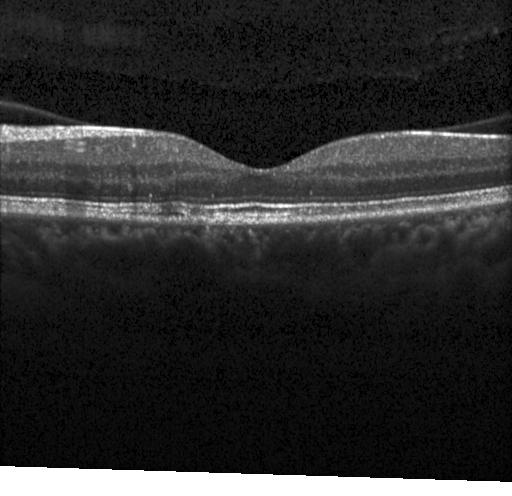

OCT finding: no choroidal neovascularization, diabetic macular edema, or drusen.